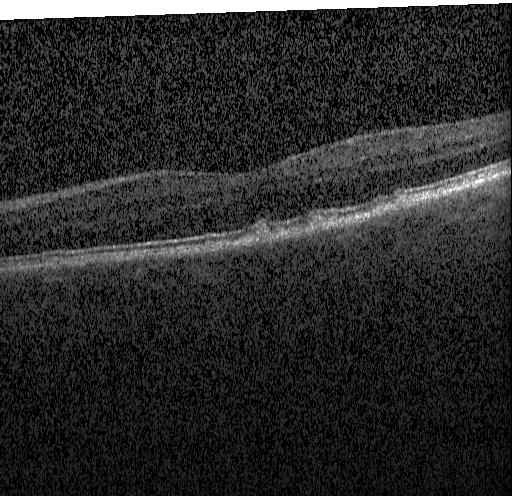

Retinal OCT B-scan, instrument: Heidelberg Spectralis. Diagnosis: multiple drusen.